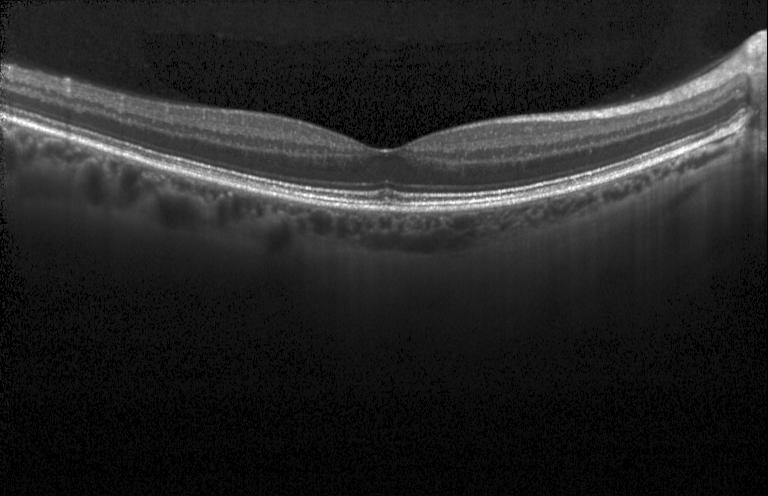

Impression: neither choroidal neovascularization, diabetic macular edema, nor drusen.